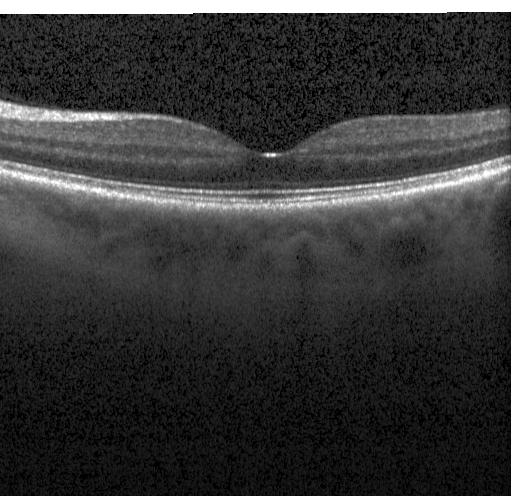

Finding: neither choroidal neovascularization, diabetic macular edema, nor drusen.